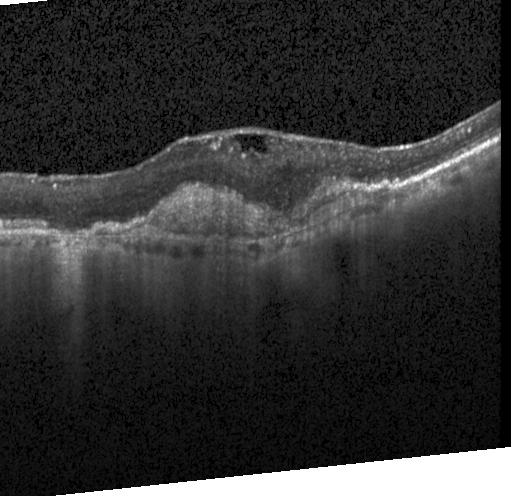
Heidelberg Spectralis · optical coherence tomography scan · SD-OCT — Diagnosis: a choroidal neovascular membrane.